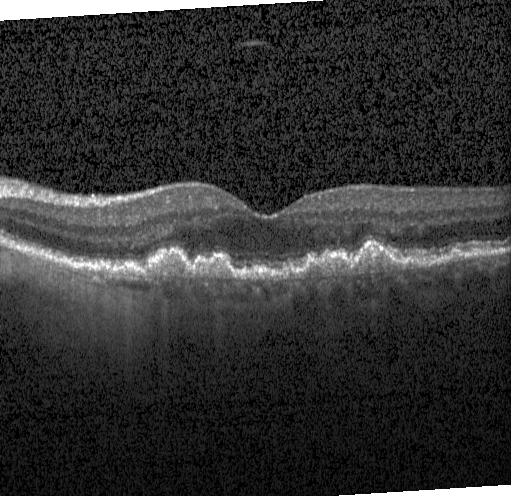

OCT line scan, through the macula, Heidelberg Spectralis
This B-scan demonstrates drusen.